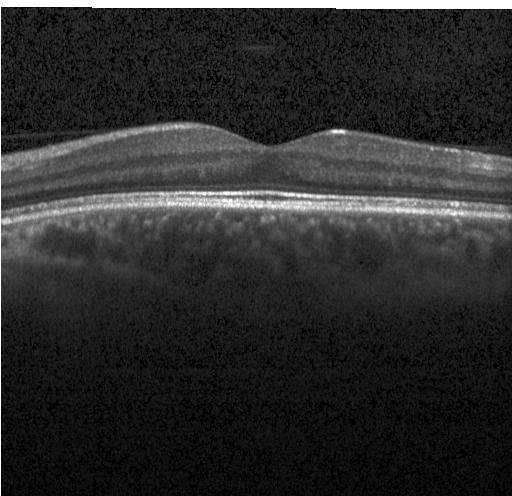 Optical coherence tomography scan; macular scan; SD-OCT; instrument: Heidelberg Spectralis. Impression: no choroidal neovascularization, diabetic macular edema, or drusen.